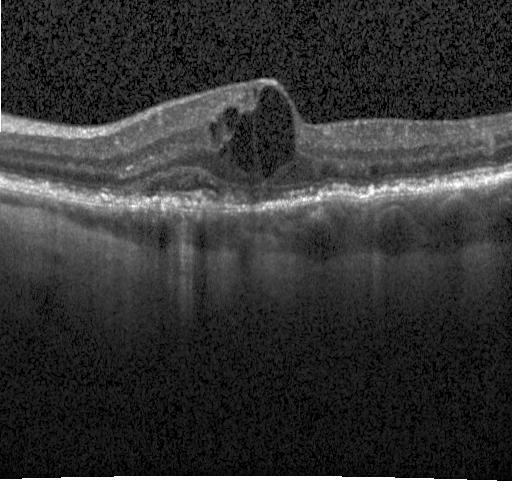
OCT B-scan; horizontal scan through the fovea; instrument: Heidelberg Spectralis
The scan shows a choroidal neovascular membrane.